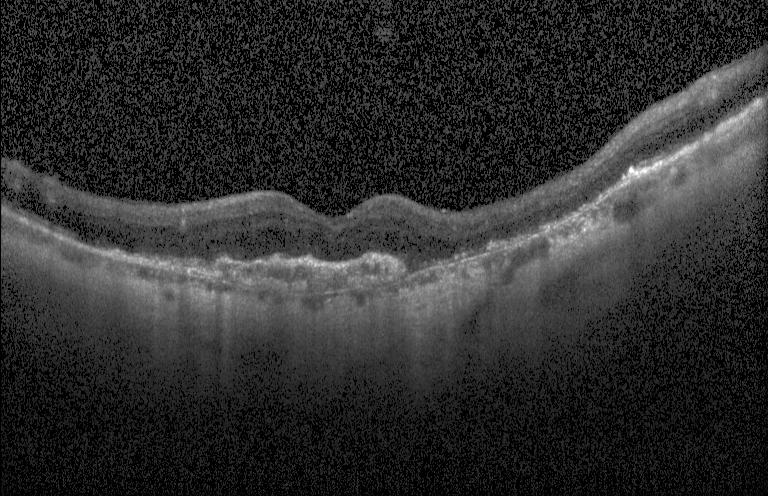 Retinal OCT cross-section, acquired on a Heidelberg Spectralis — Diagnosis: choroidal neovascularization.